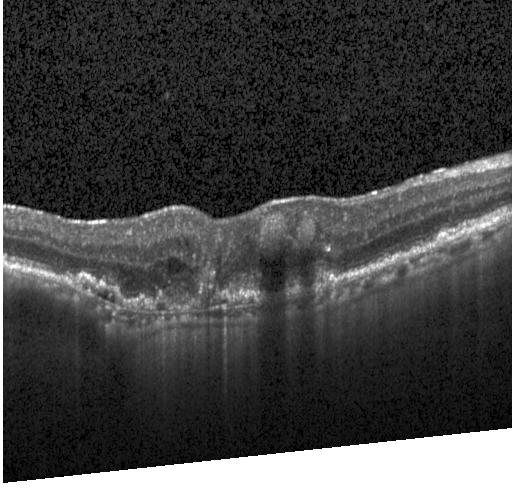

The scan shows choroidal neovascularization.